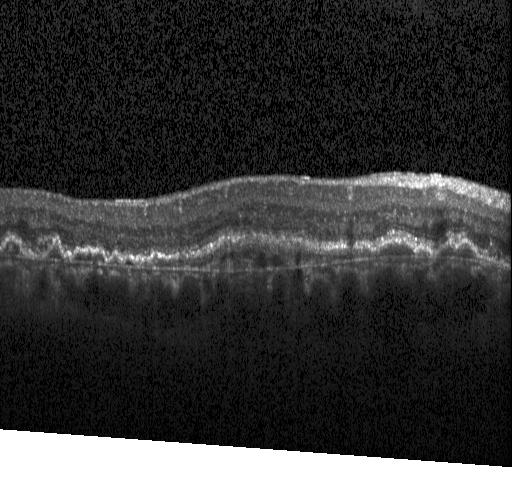
Retinal OCT cross-section, spectral-domain OCT — Diagnosis: CNV.